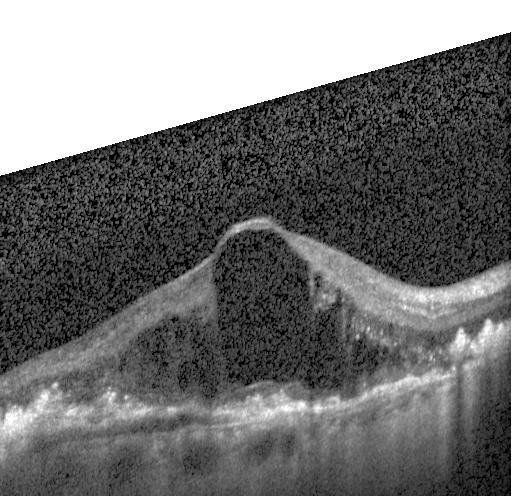 A choroidal neovascular membrane.